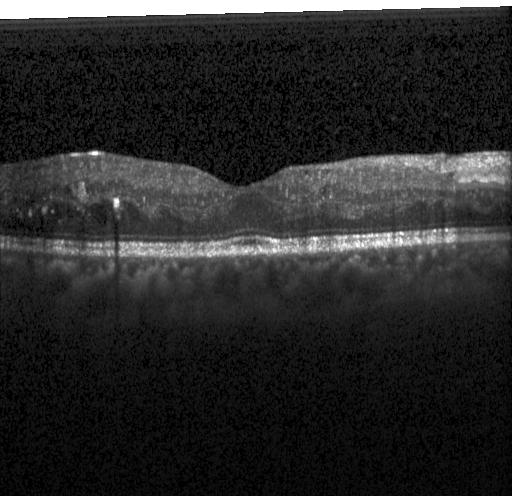

Retinal OCT B-scan, horizontal scan through the fovea, spectral-domain optical coherence tomography. Diagnosis: diabetic macular edema.